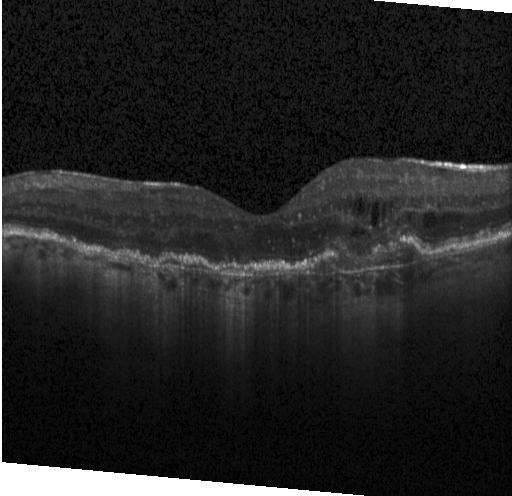

Optical coherence tomography scan — The scan shows CNV.